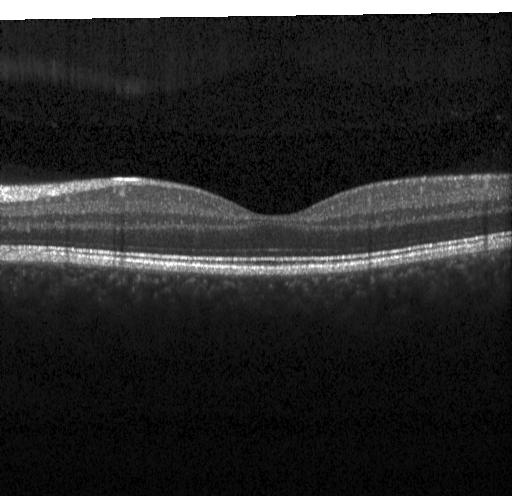
Spectral-domain OCT. Optical coherence tomography B-scan — No choroidal neovascularization, no diabetic macular edema, and no drusen.